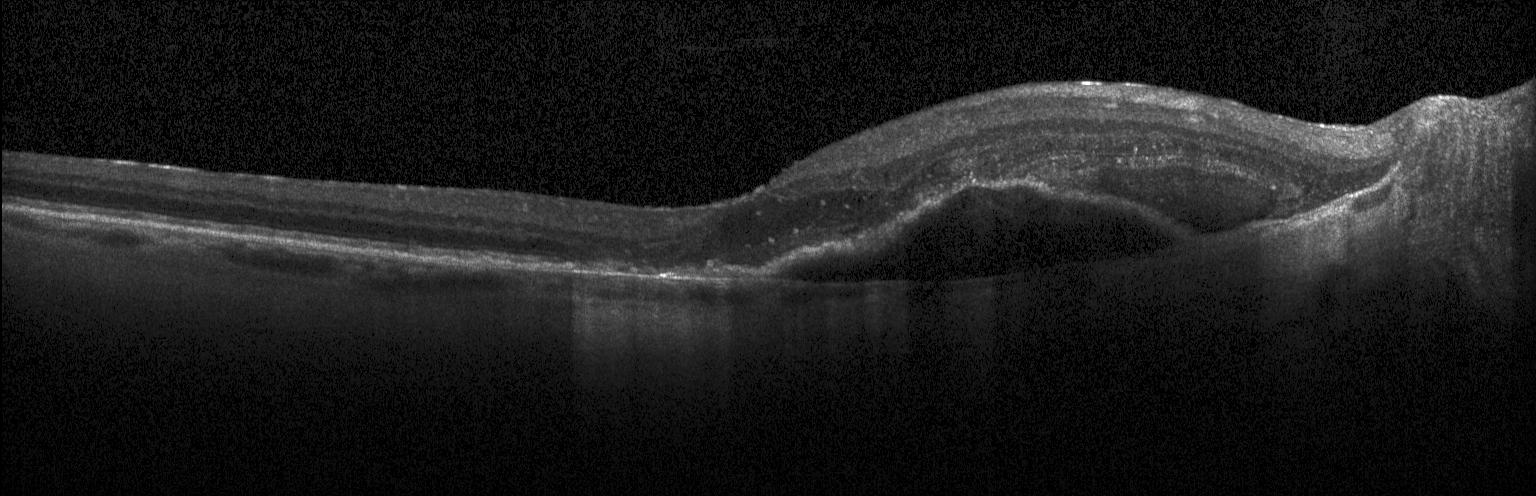
Impression: CNV.